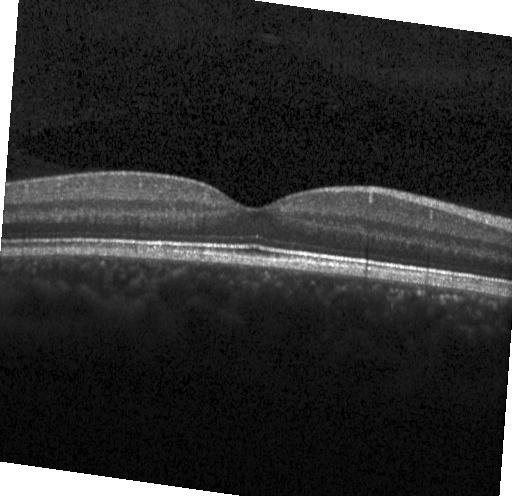

Centered on the fovea. Heidelberg Spectralis OCT system. Spectral-domain optical coherence tomography. OCT B-scan
Finding: no evidence of choroidal neovascularization, diabetic macular edema, or drusen.